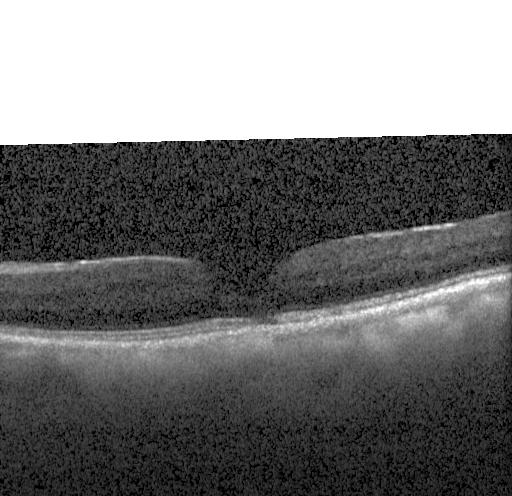

Macular OCT: no CNV, no DME, and no drusen.